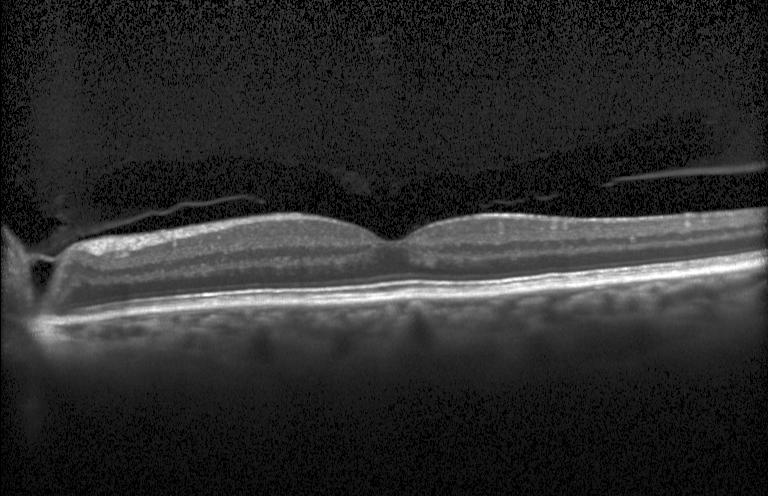
Heidelberg Spectralis; macular scan; optical coherence tomography B-scan. Impression: no CNV, DME, or drusen.